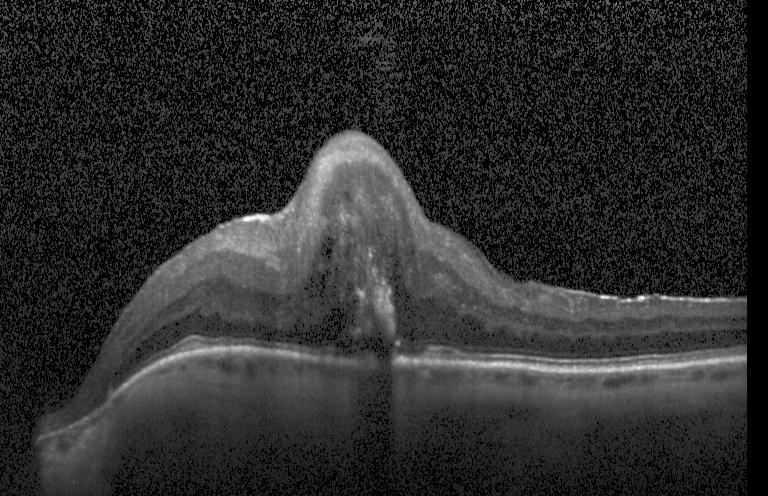

A choroidal neovascular membrane.